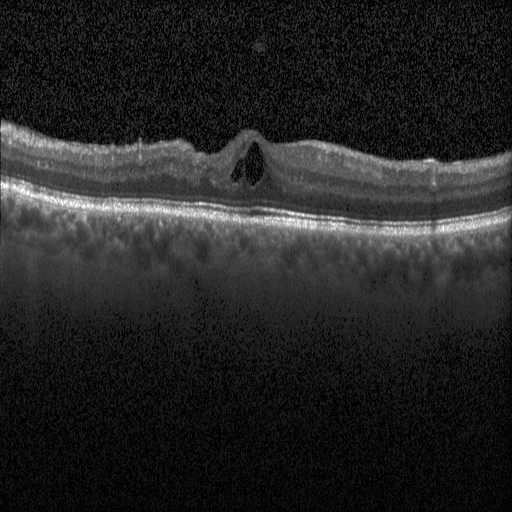

OCT B-scan
OCT finding: DME.